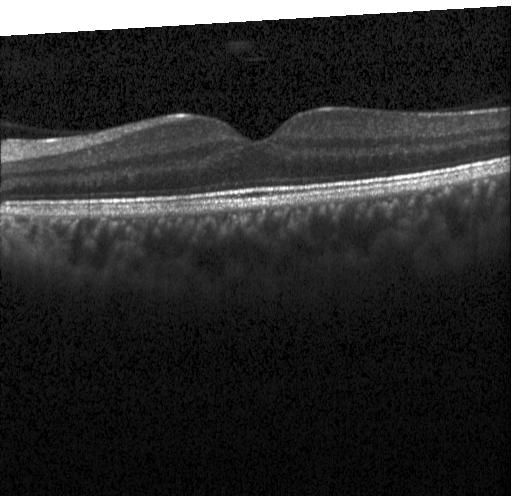

OCT finding: no evidence of choroidal neovascularization, diabetic macular edema, or drusen.